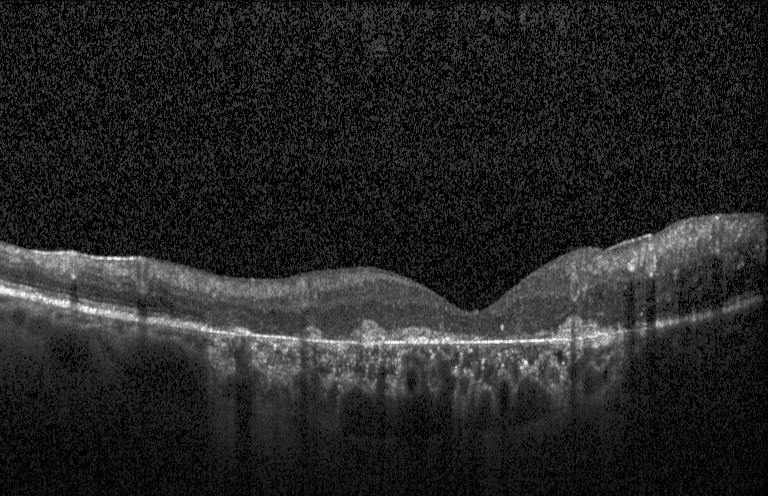
Heidelberg Spectralis · spectral-domain OCT · retinal OCT cross-section — Macular OCT: a choroidal neovascular membrane.